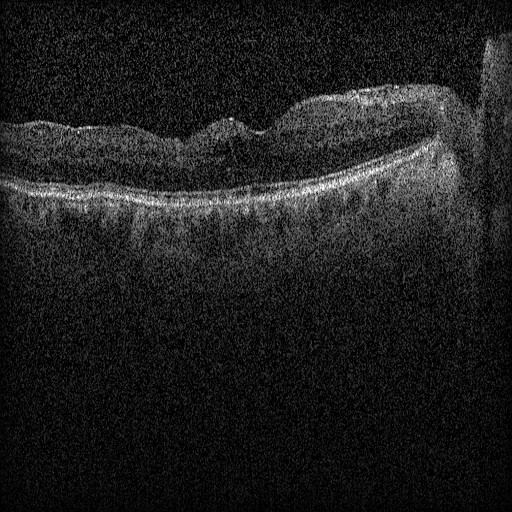 OCT B-scan — Finding: DME.